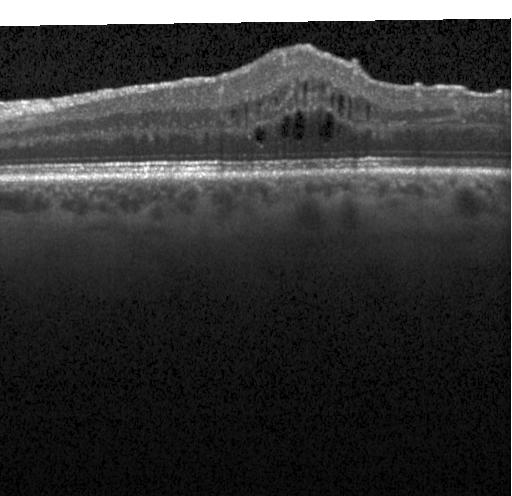 Impression: diabetic macular edema.